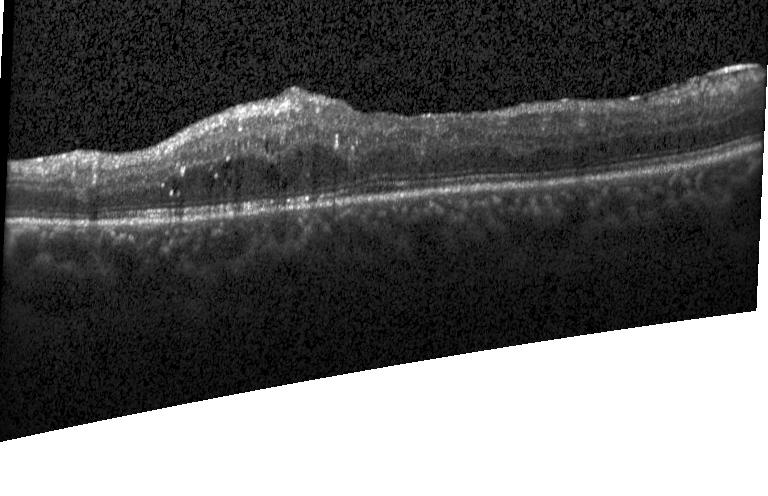

Impression: diabetic macular edema (DME).